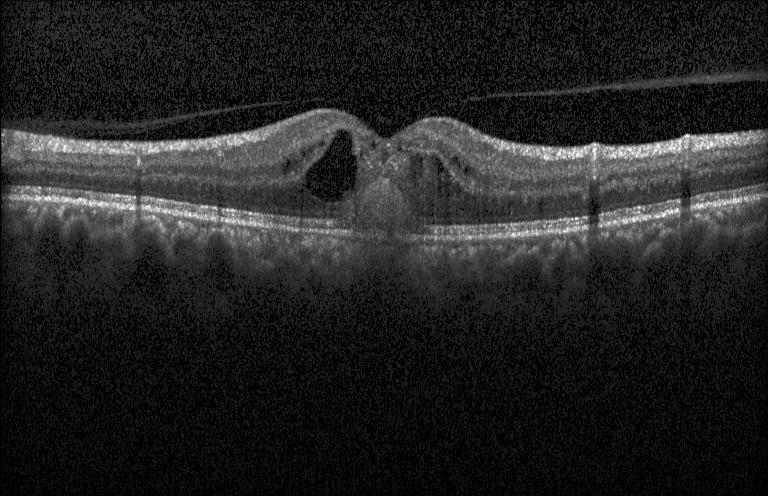 Optical coherence tomography B-scan. Assessment: a choroidal neovascular membrane.